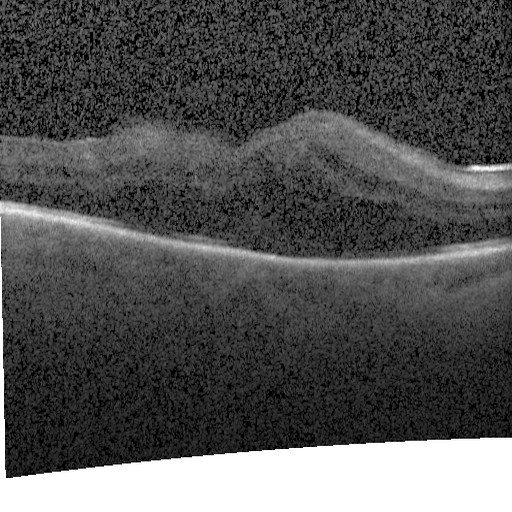

Macular OCT demonstrating diabetic macular edema.